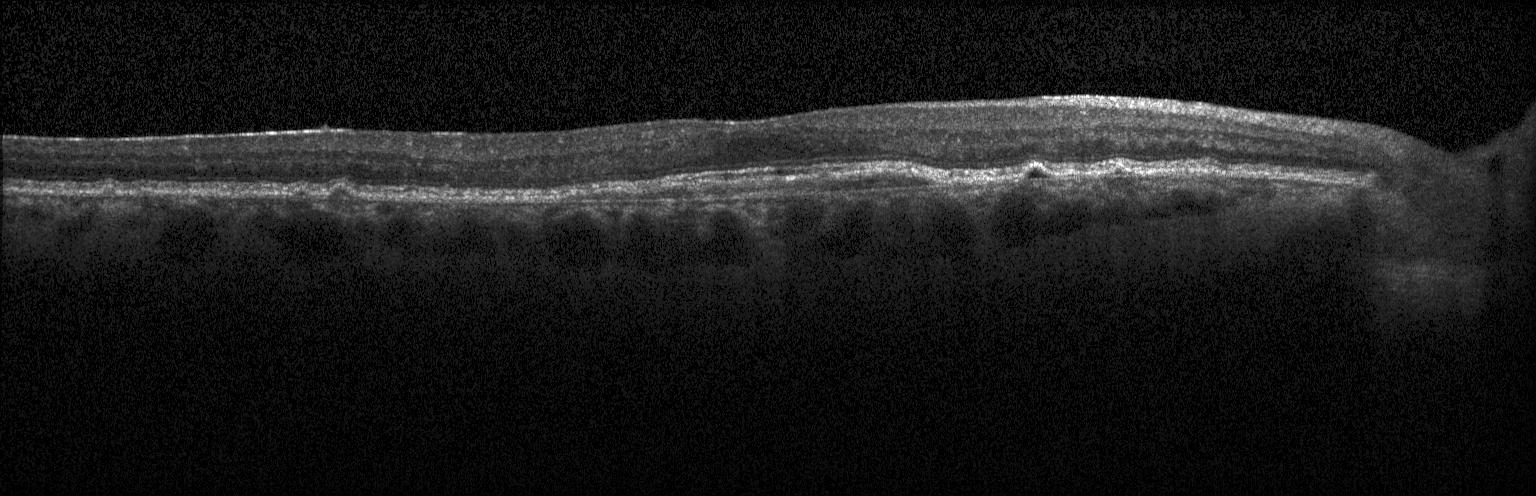

OCT line scan. The scan shows a choroidal neovascular membrane.